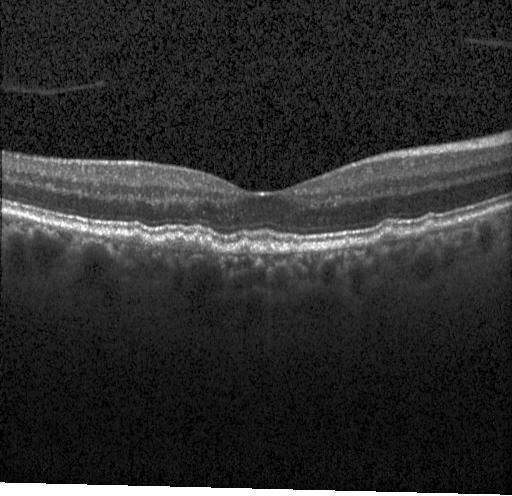

Optical coherence tomography scan; macular scan; spectral-domain OCT — Assessment: sub-RPE drusenoid deposits.